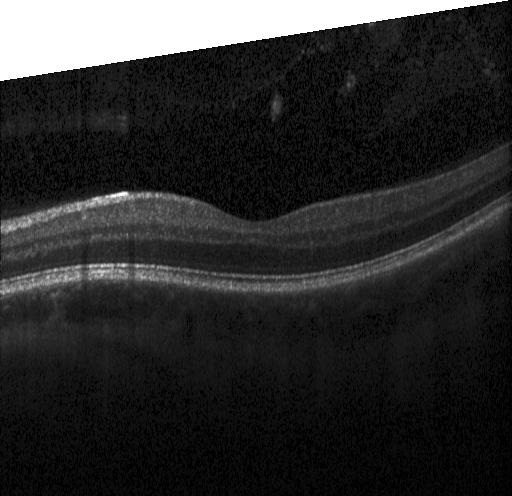

OCT scan showing neither choroidal neovascularization, diabetic macular edema, nor drusen.